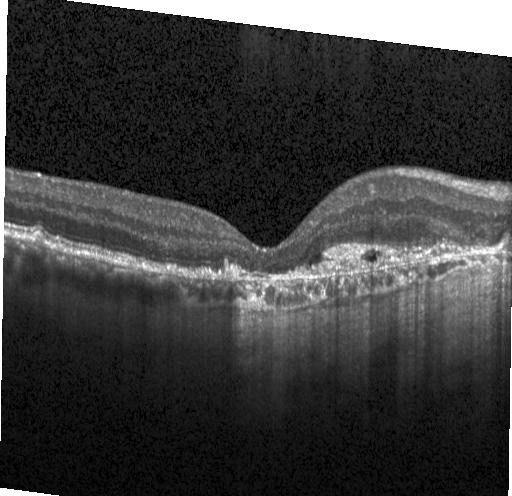
Through the macula · spectral-domain optical coherence tomography · instrument: Heidelberg Spectralis · retinal OCT B-scan.
Dx: choroidal neovascularization.